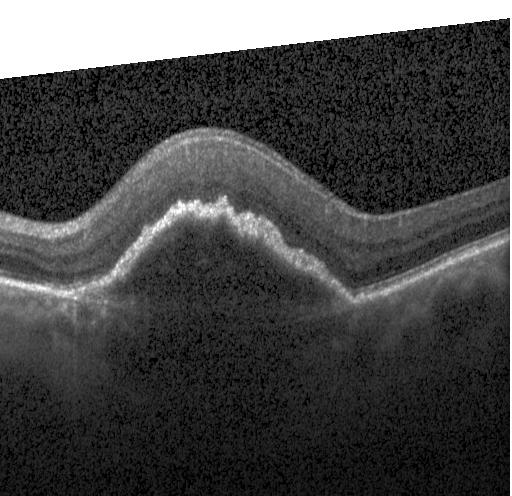
Horizontal scan through the fovea · retinal OCT cross-section · acquired on a Heidelberg Spectralis
Dx: choroidal neovascularization.